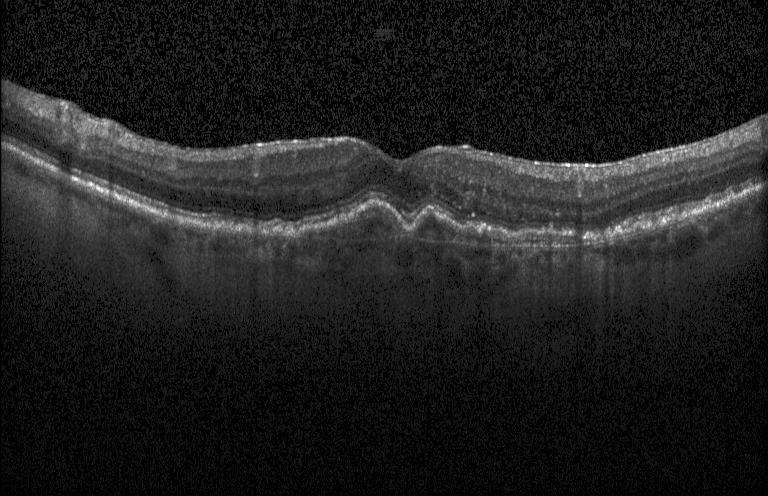
OCT B-scan. Assessment: a choroidal neovascular membrane.